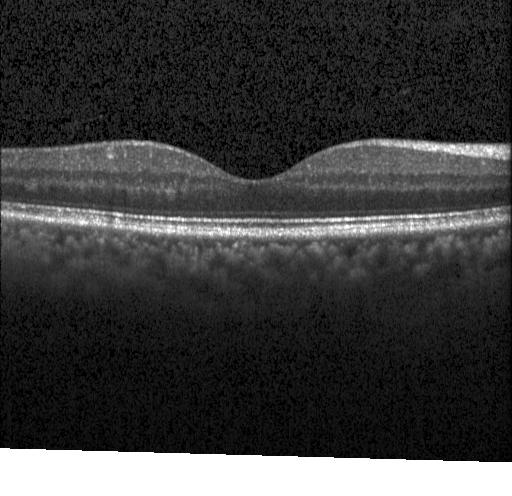
OCT B-scan showing no evidence of choroidal neovascularization, diabetic macular edema, or drusen.